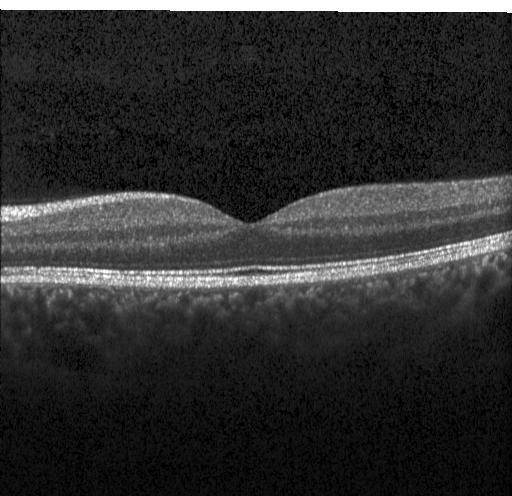 Finding: no evidence of choroidal neovascularization, diabetic macular edema, or drusen.